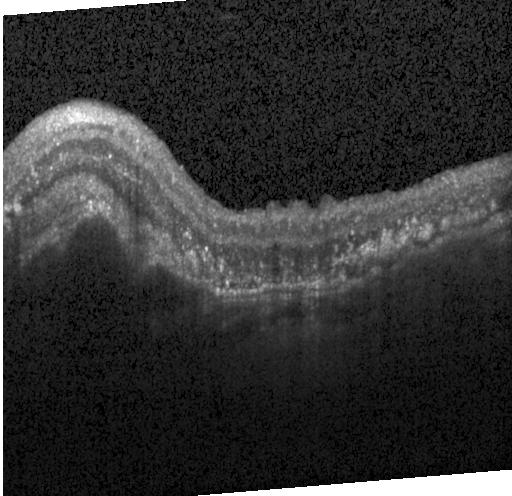
Optical coherence tomography scan · centered on the fovea
Diagnosis: CNV.